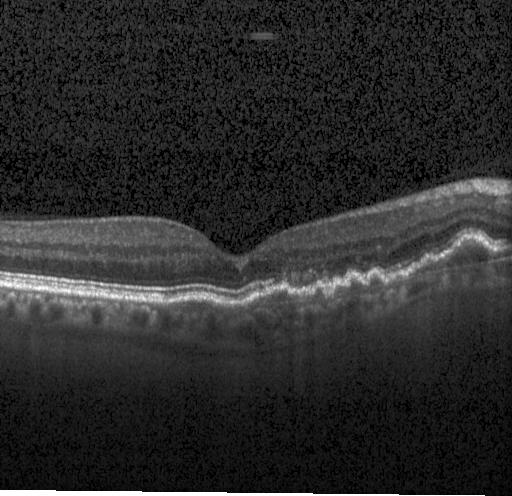

OCT B-scan showing a choroidal neovascular membrane.